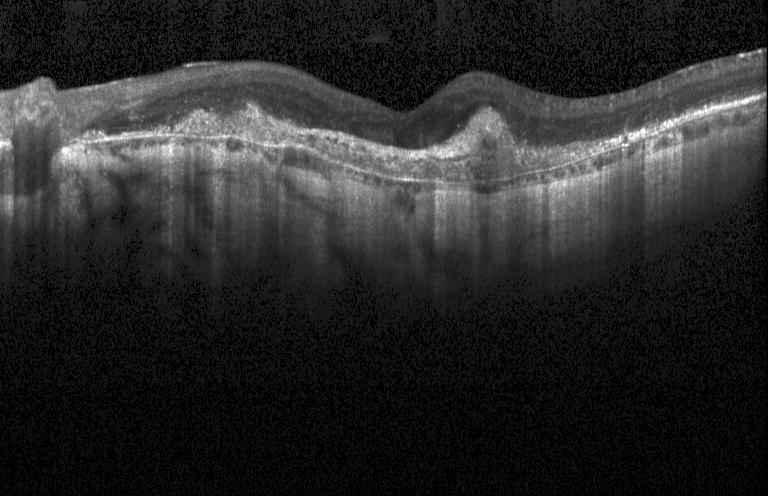
Acquired on a Heidelberg Spectralis, retinal OCT cross-section. Impression: CNV.